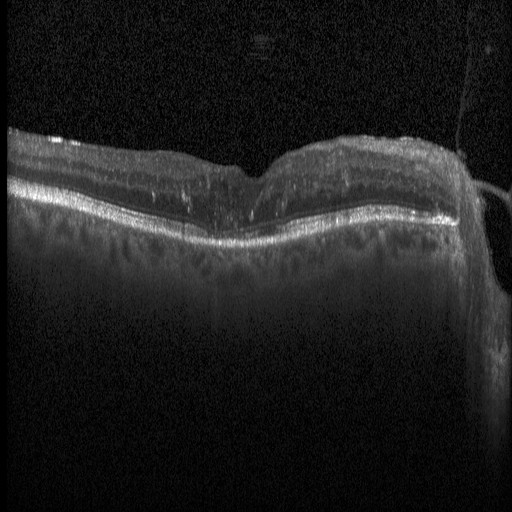
Macular scan, optical coherence tomography scan, Heidelberg Spectralis, spectral-domain optical coherence tomography
DME.